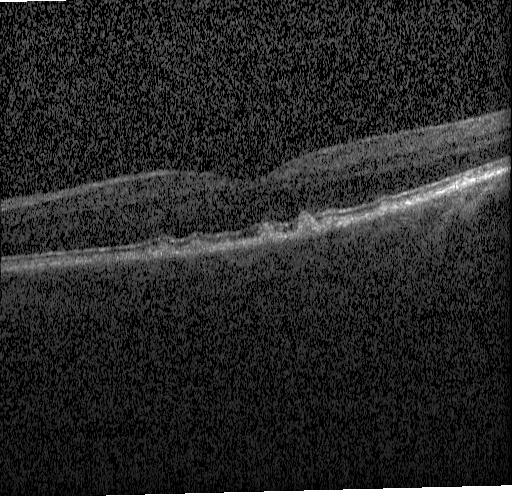
Retinal OCT cross-section. SD-OCT. Heidelberg Spectralis OCT system. Centered on the fovea. Macular OCT: sub-RPE drusenoid deposits.